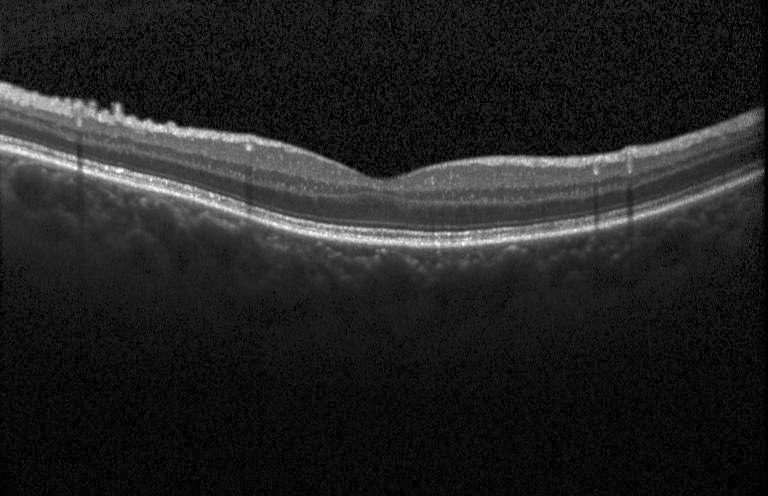 SD-OCT, instrument: Heidelberg Spectralis, optical coherence tomography B-scan — No evidence of choroidal neovascularization, diabetic macular edema, or drusen.